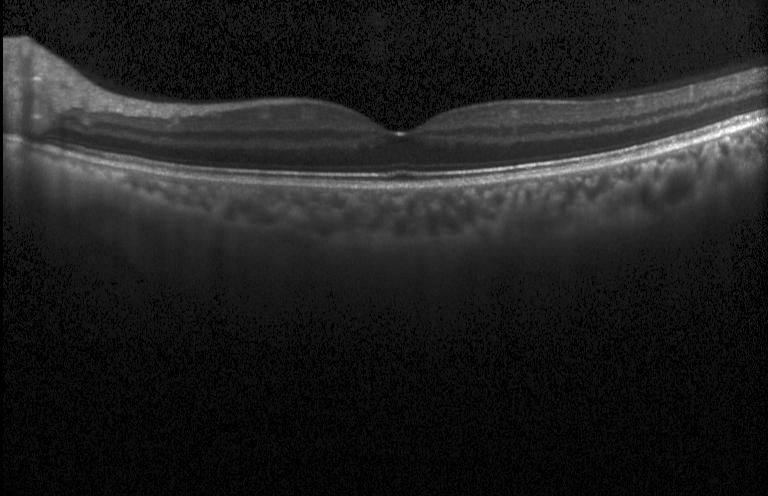
Macular OCT demonstrating no CNV, no DME, and no drusen.